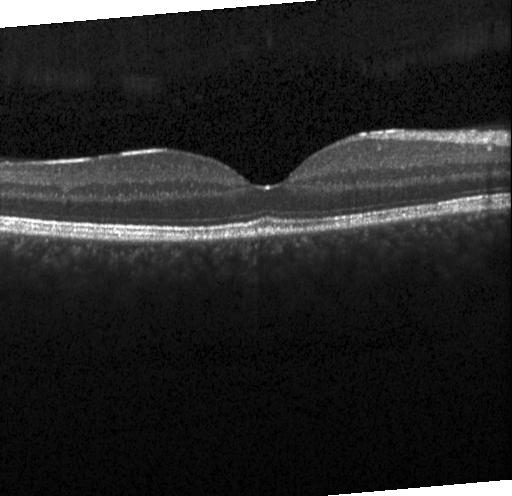

Retinal OCT B-scan — Dx: neither choroidal neovascularization, diabetic macular edema, nor drusen.